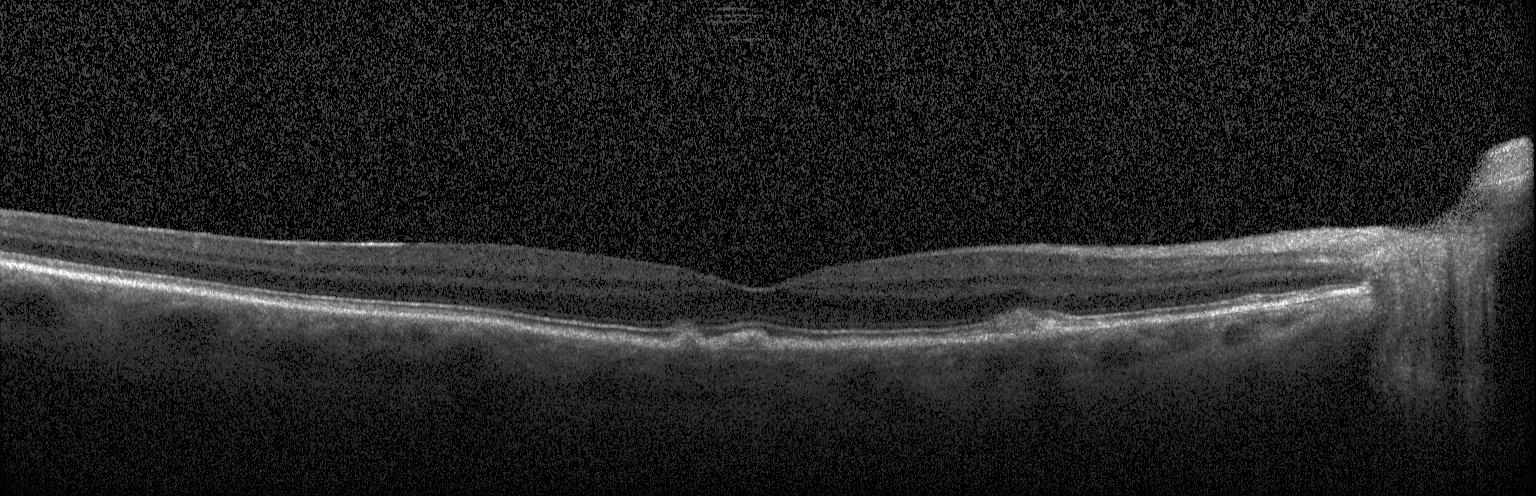

OCT line scan
Finding: sub-RPE drusenoid deposits.